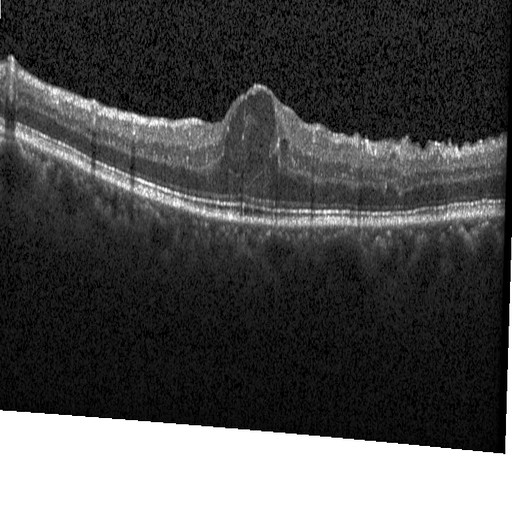 Optical coherence tomography B-scan
The scan shows diabetic macular edema (DME).